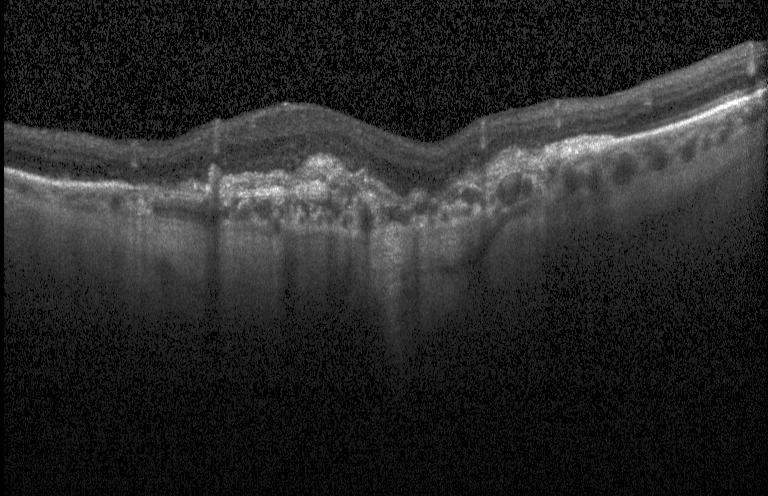
Retinal OCT B-scan. Diagnosis: choroidal neovascularization.